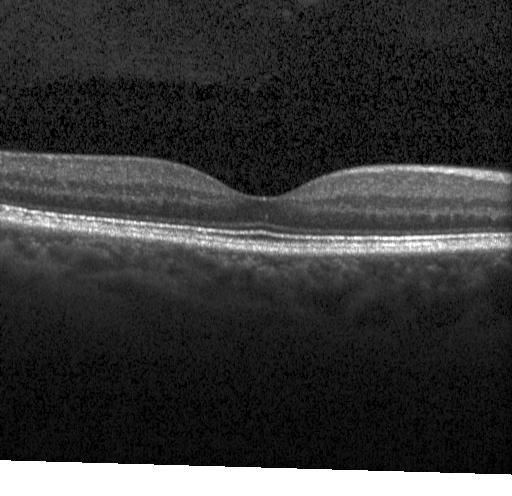

Dx: no CNV, no DME, and no drusen.